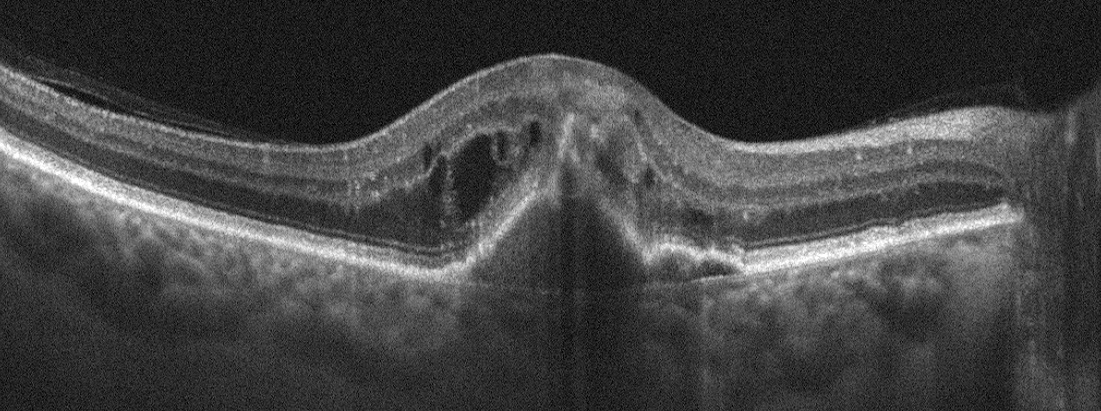
Spectral-domain OCT B-scan: AMD.